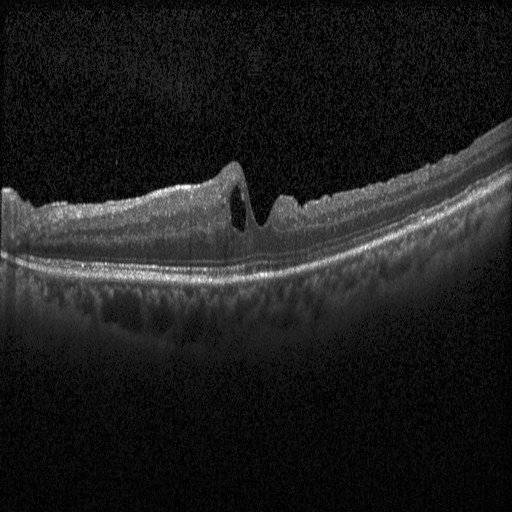 Macular OCT demonstrating diabetic macular edema.